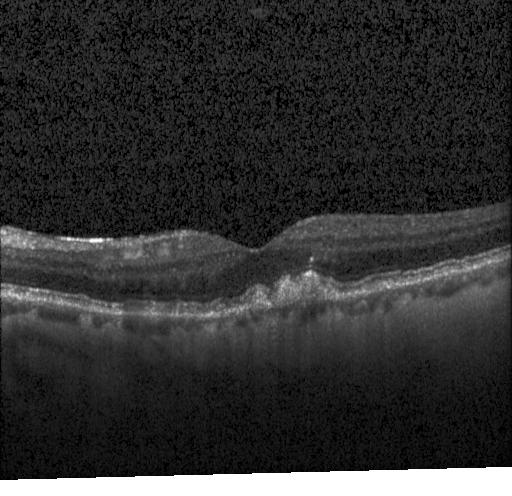 Macular OCT: drusen.